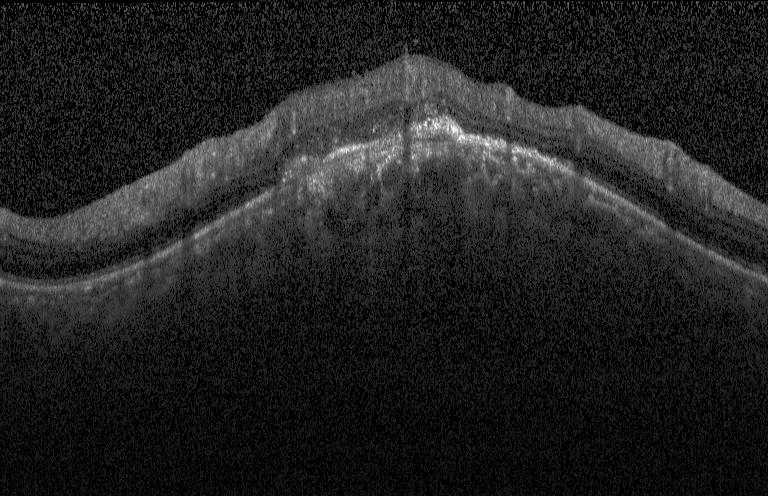 Macular scan; retinal OCT cross-section; Heidelberg Spectralis OCT system. This B-scan demonstrates a choroidal neovascular membrane.